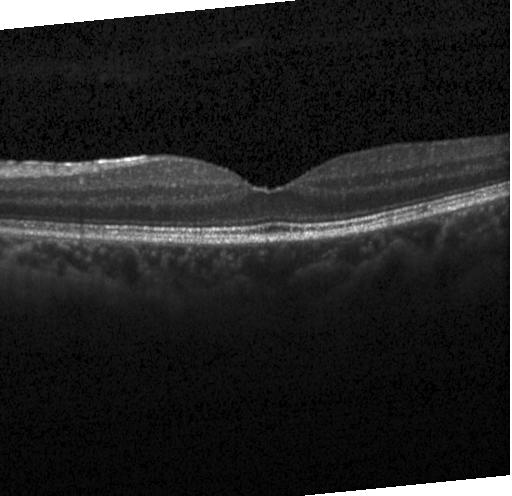
Fovea-centered; Heidelberg Spectralis OCT system; spectral-domain optical coherence tomography; retinal OCT B-scan
No choroidal neovascularization, no diabetic macular edema, and no drusen.